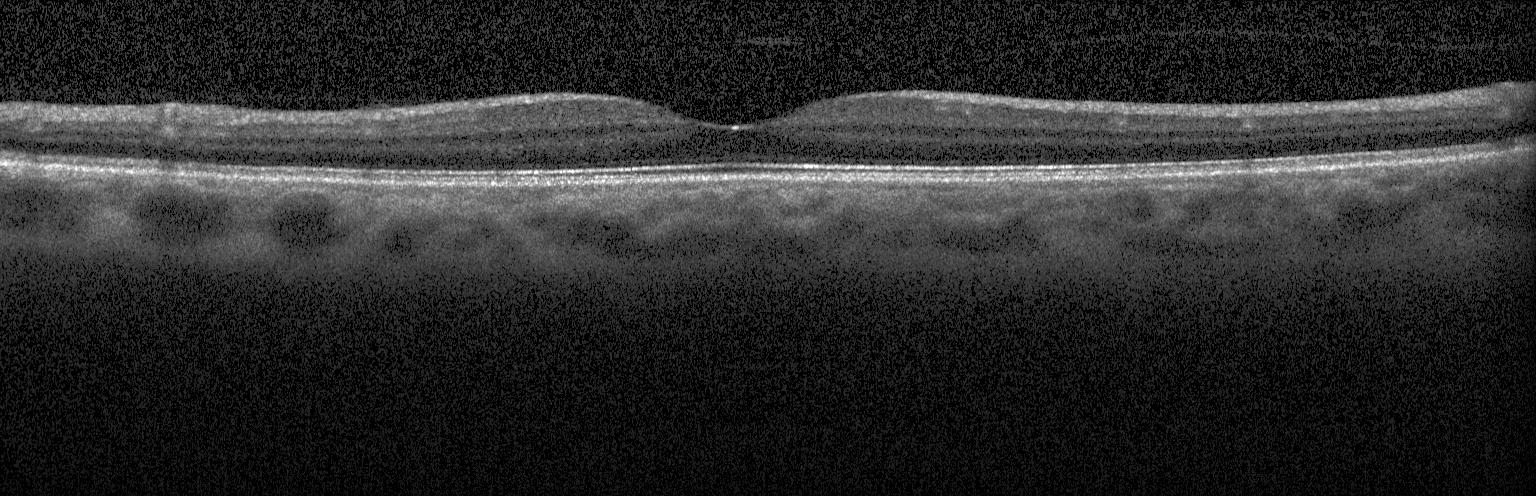 Optical coherence tomography scan
Assessment: no evidence of CNV, DME, or drusen.